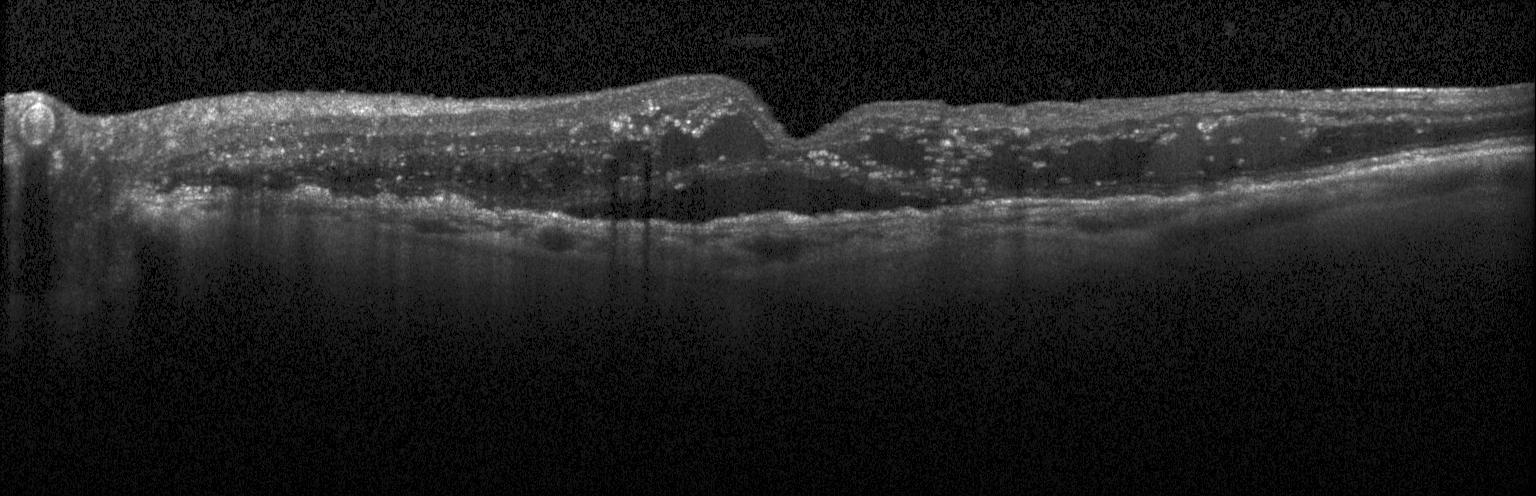

Macular scan. Retinal OCT B-scan. Diagnosis: a choroidal neovascular membrane.